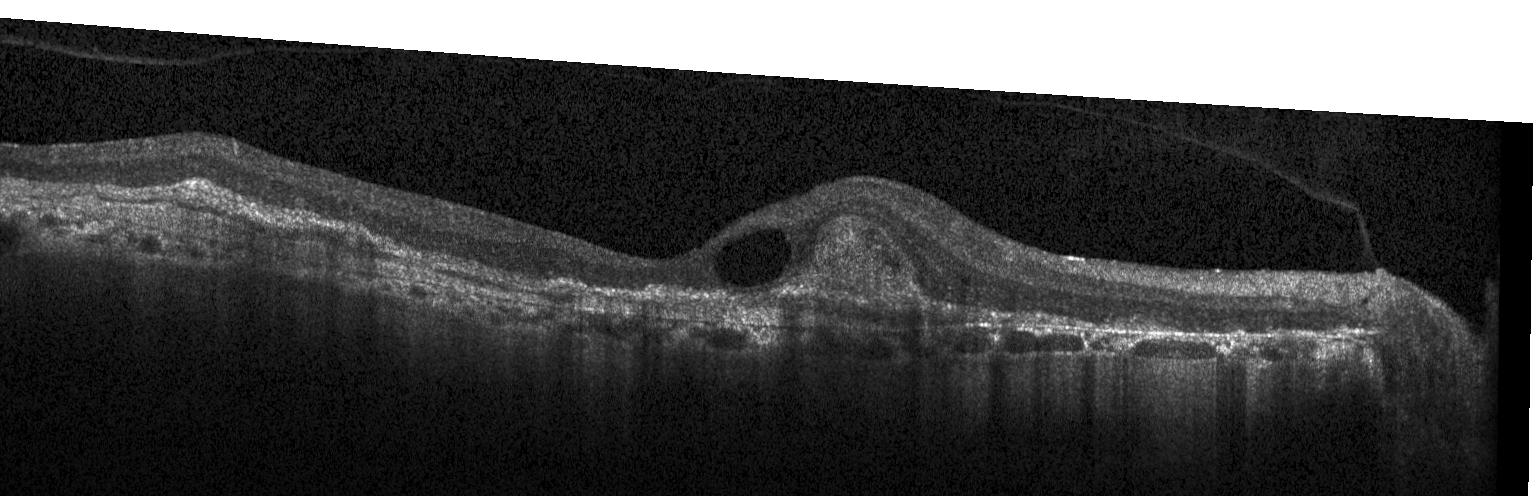 Impression: a choroidal neovascular membrane.